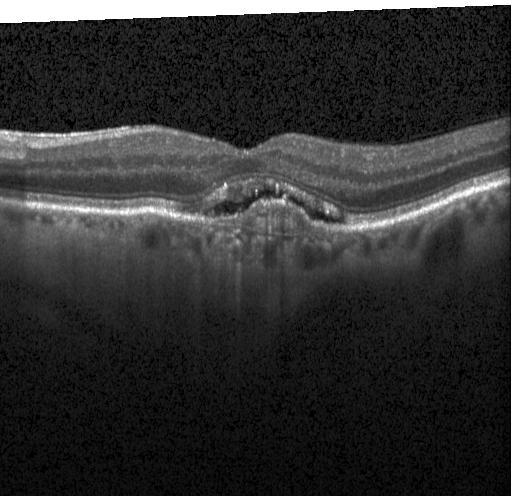 Acquired on a Heidelberg Spectralis; OCT line scan — A choroidal neovascular membrane.